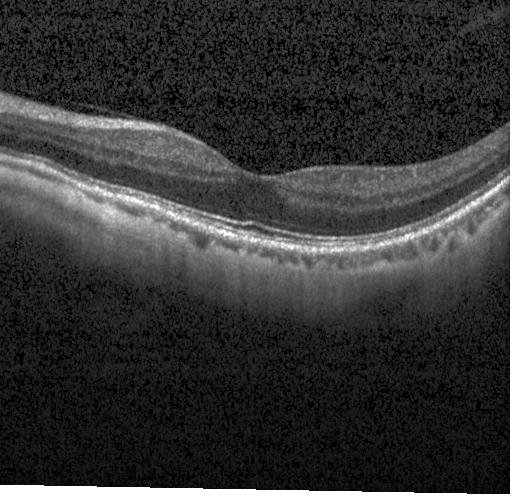

Spectral-domain OCT. Optical coherence tomography B-scan. Acquired on a Heidelberg Spectralis. No evidence of CNV, DME, or drusen.